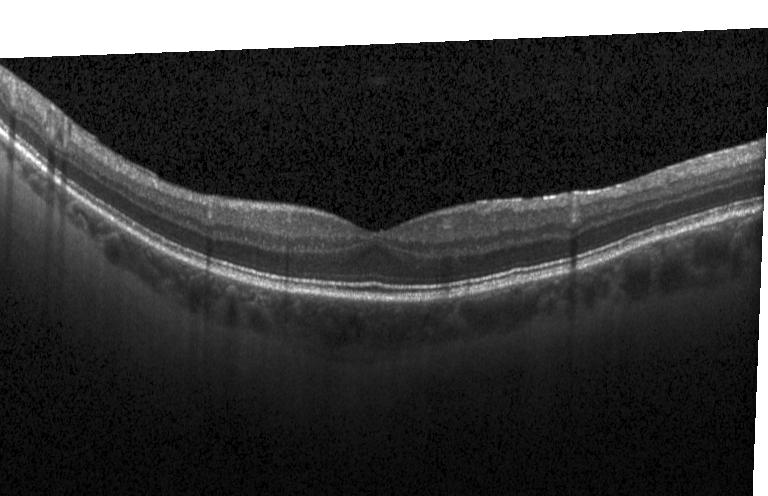 Optical coherence tomography scan · Heidelberg Spectralis · horizontal scan through the fovea · spectral-domain optical coherence tomography.
Finding: no choroidal neovascularization, diabetic macular edema, or drusen.